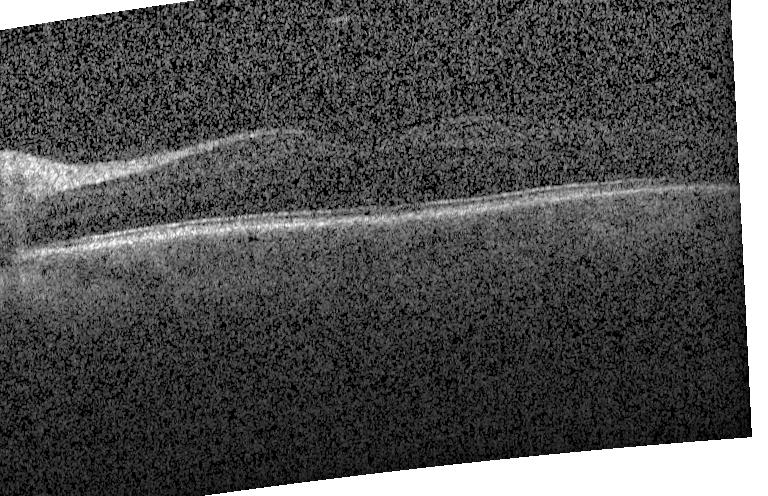

Diagnosis: no choroidal neovascularization, diabetic macular edema, or drusen.